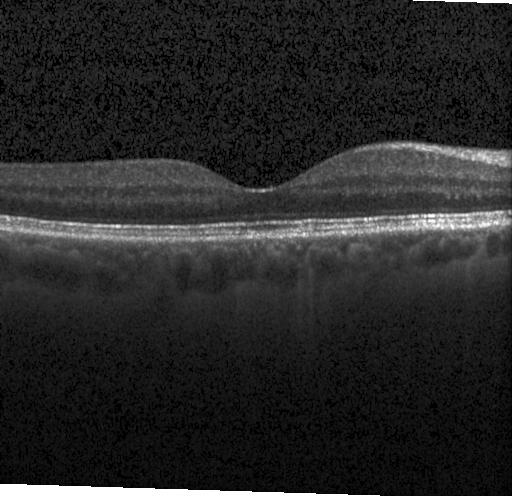
Acquired on a Heidelberg Spectralis; SD-OCT; optical coherence tomography B-scan — Diagnosis: no choroidal neovascularization, diabetic macular edema, or drusen.